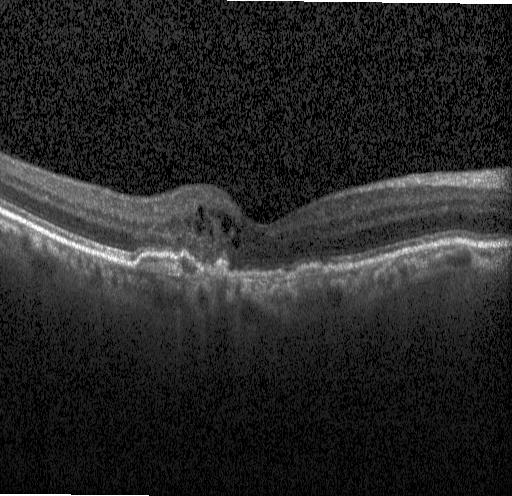 Optical coherence tomography scan; Heidelberg Spectralis OCT system
This B-scan demonstrates CNV.